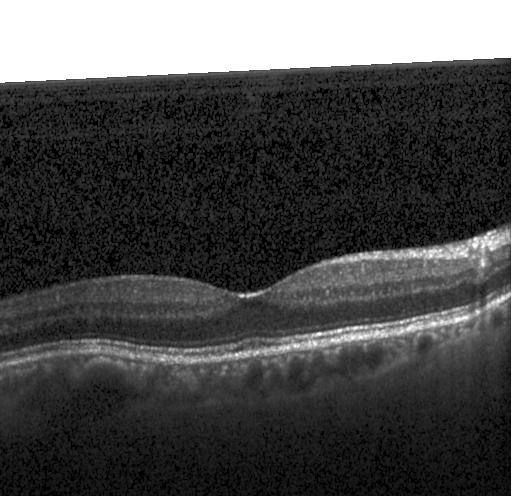

Retinal OCT cross-section — The scan shows no choroidal neovascularization, no diabetic macular edema, and no drusen.